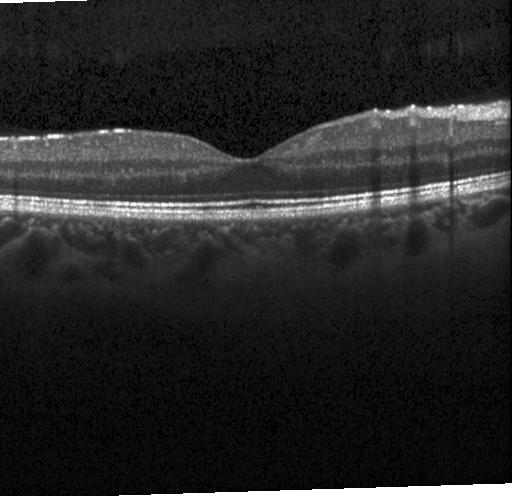

Assessment: no CNV, DME, or drusen.